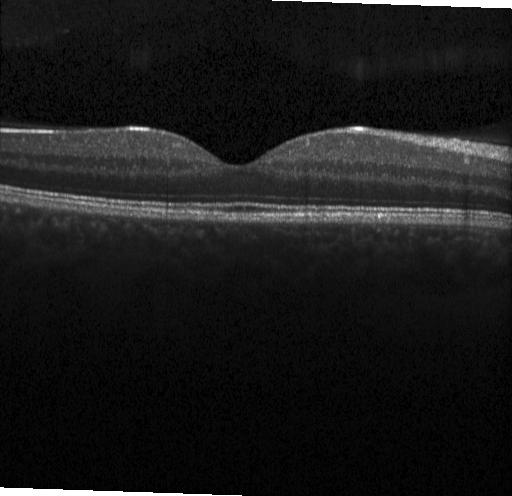
Diagnosis: no choroidal neovascularization, no diabetic macular edema, and no drusen.